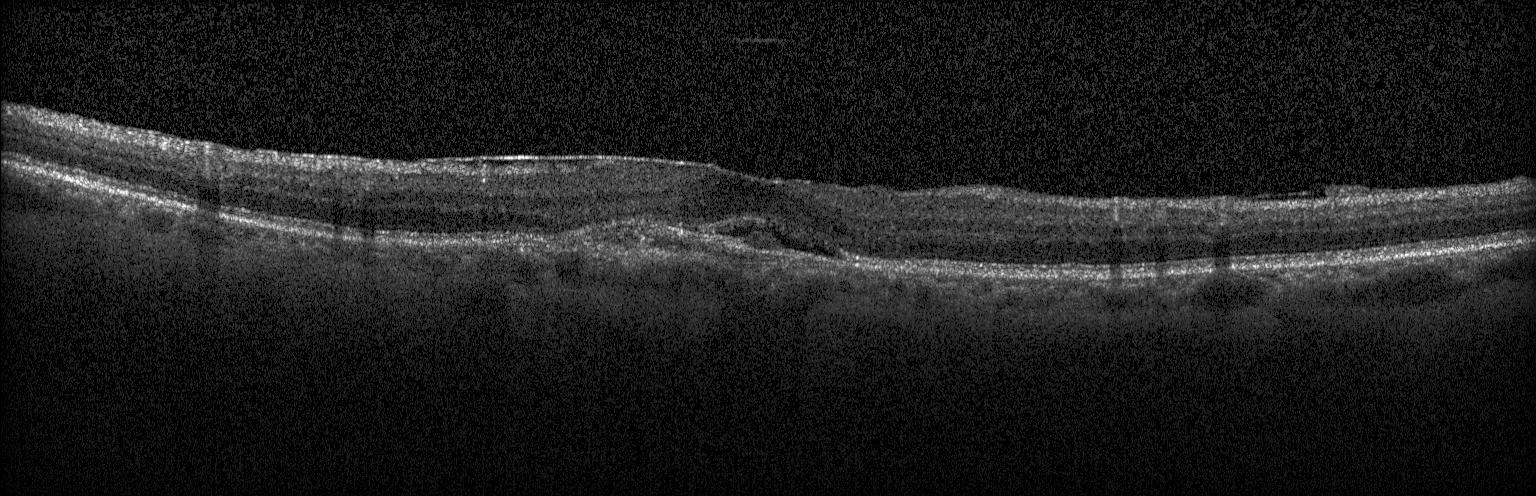
OCT scan showing choroidal neovascularization (CNV).